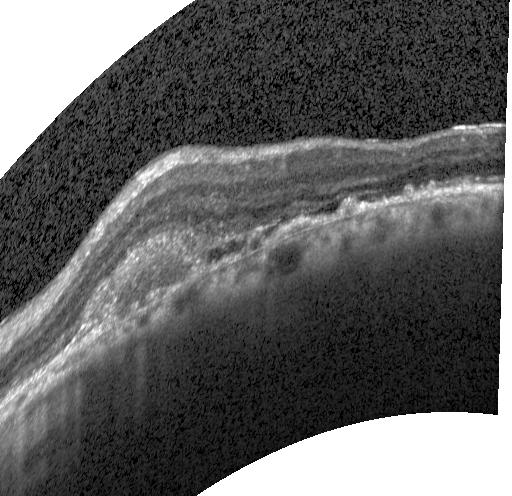
Spectral-domain OCT · retinal OCT B-scan · Heidelberg Spectralis · horizontal scan through the fovea. This B-scan demonstrates a choroidal neovascular membrane.